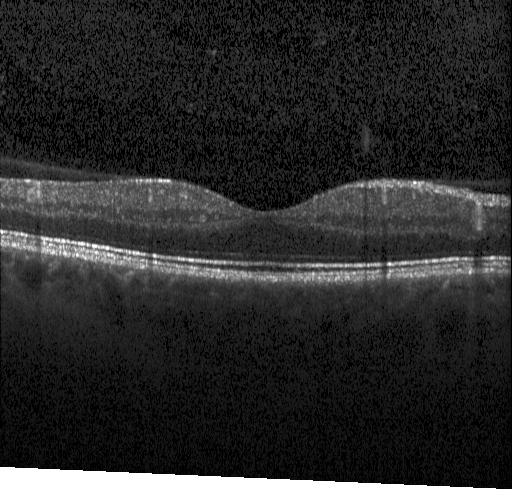

Impression: neither CNV, DME, nor drusen.